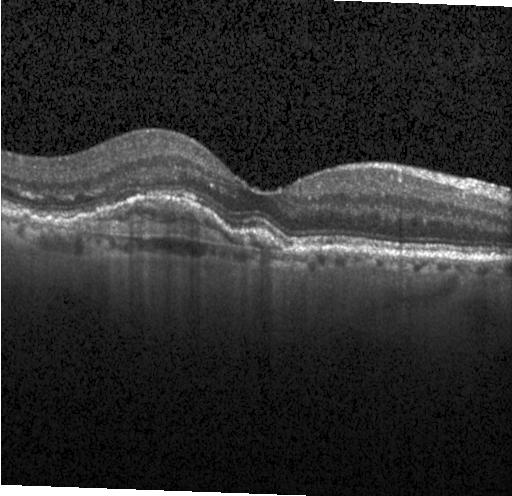
Instrument: Heidelberg Spectralis · OCT line scan. The scan shows choroidal neovascularization.